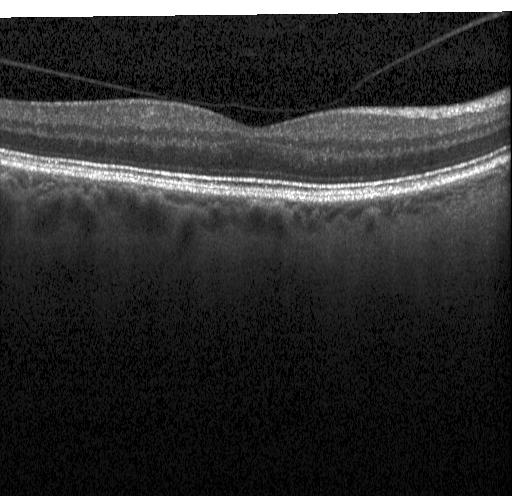

OCT line scan. Centered on the fovea. Spectral-domain OCT.
This B-scan demonstrates no choroidal neovascularization, no diabetic macular edema, and no drusen.